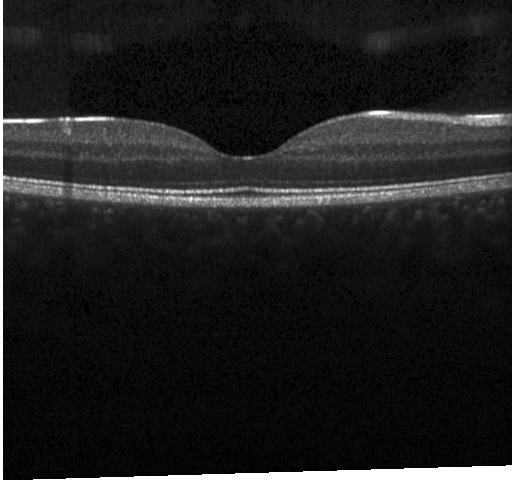

Impression: no choroidal neovascularization, no diabetic macular edema, and no drusen.